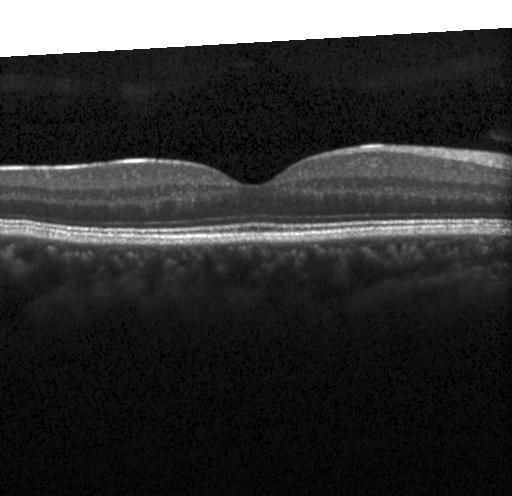

Spectral-domain OCT B-scan: no evidence of choroidal neovascularization, diabetic macular edema, or drusen.